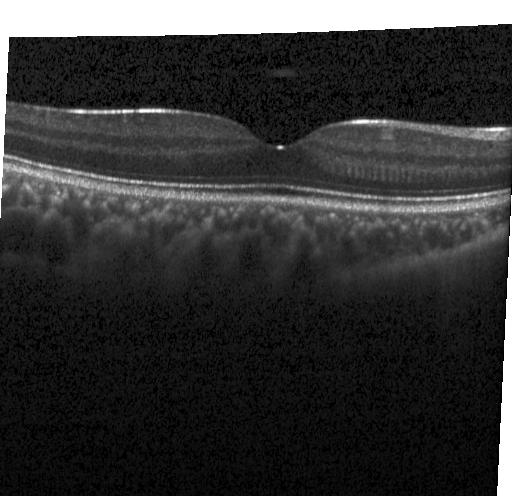

Spectral-domain OCT B-scan: neither choroidal neovascularization, diabetic macular edema, nor drusen.